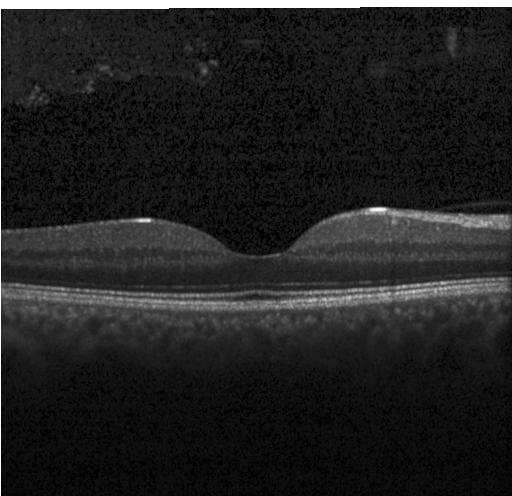 Dx: no CNV, no DME, and no drusen.